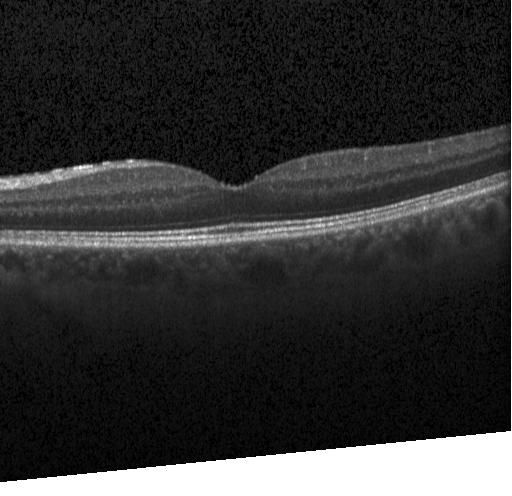

Macular OCT demonstrating neither CNV, DME, nor drusen.